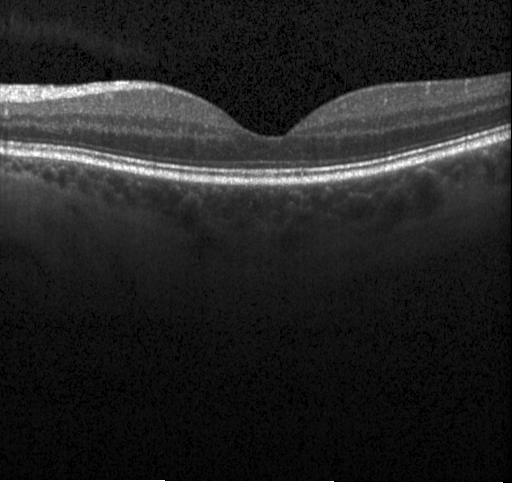
Diagnosis: no choroidal neovascularization, diabetic macular edema, or drusen.